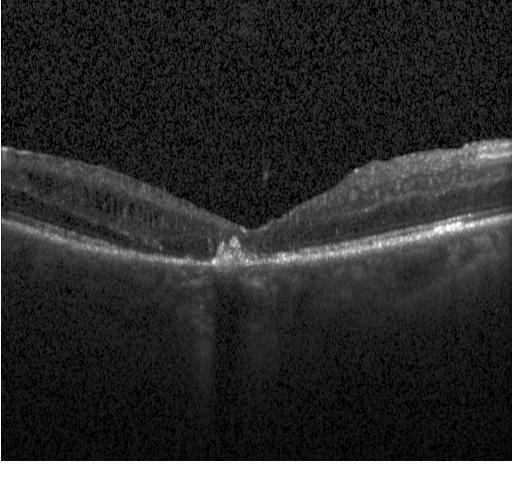 OCT line scan. Diagnosis: choroidal neovascularization.